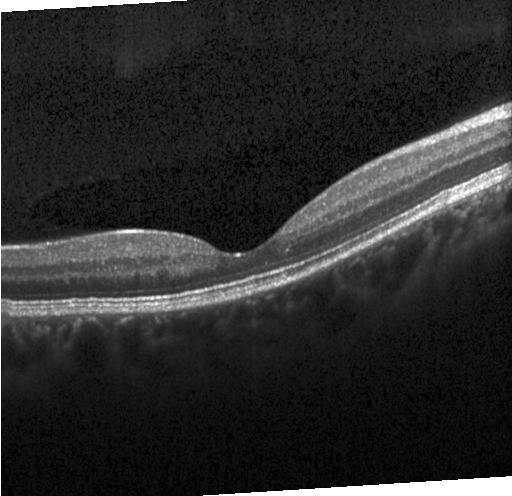

Instrument: Heidelberg Spectralis; spectral-domain optical coherence tomography; optical coherence tomography B-scan — Diagnosis: no choroidal neovascularization, no diabetic macular edema, and no drusen.